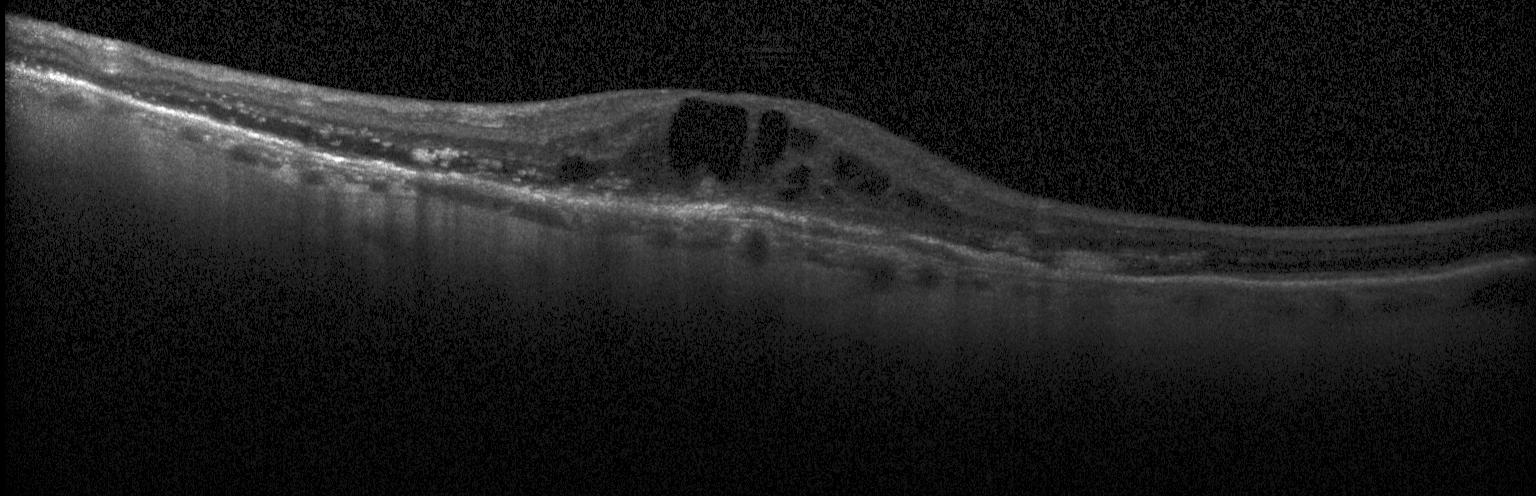

Acquired on a Heidelberg Spectralis, optical coherence tomography B-scan — OCT finding: choroidal neovascularization (CNV).